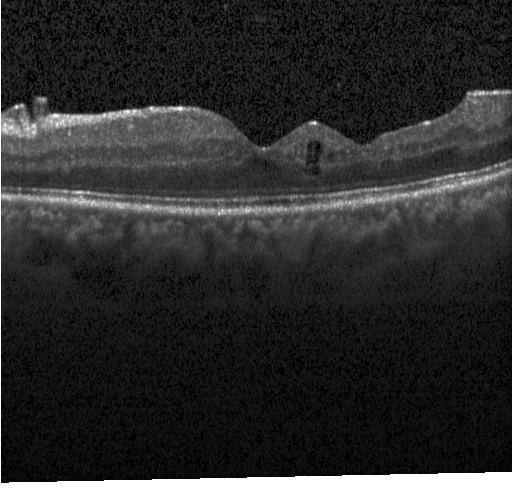
The scan shows diabetic macular edema.